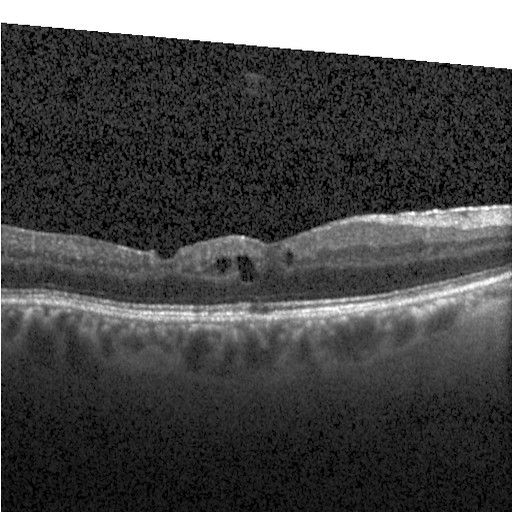
OCT scan showing diabetic macular edema.